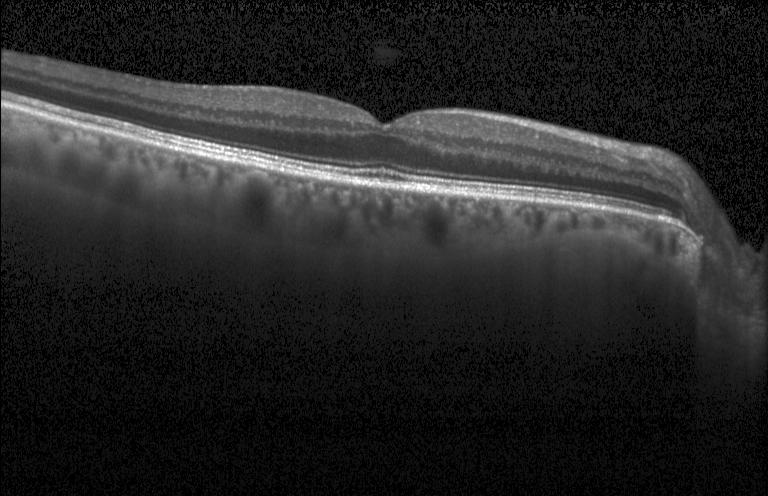

OCT finding: no evidence of choroidal neovascularization, diabetic macular edema, or drusen.